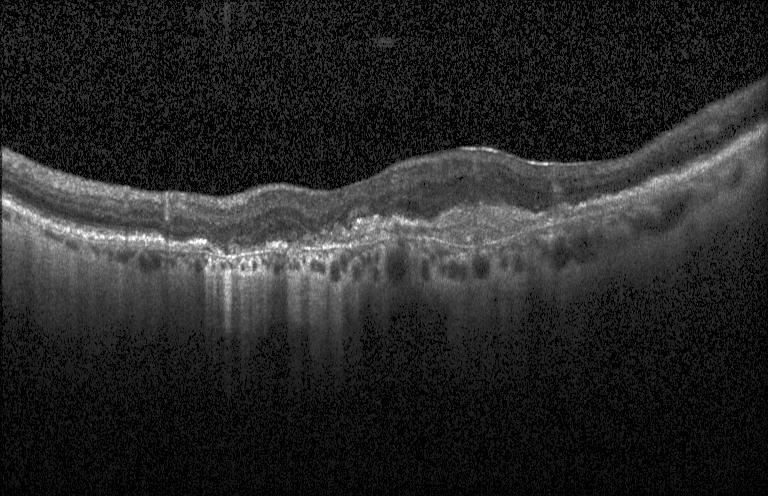
A choroidal neovascular membrane.